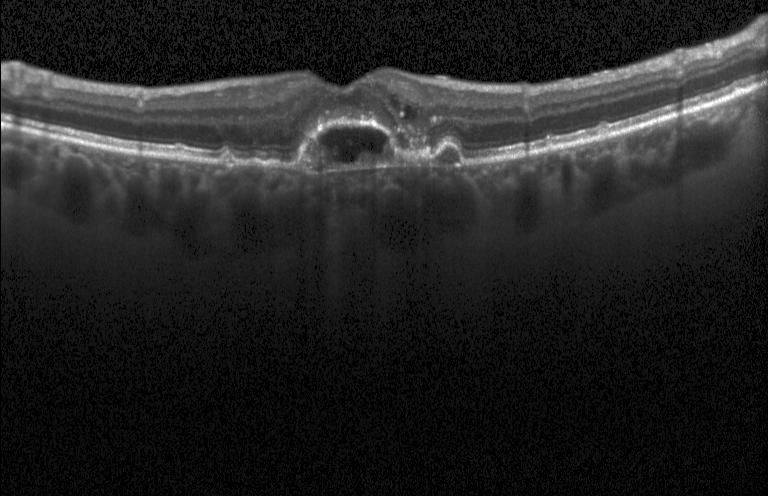 Macular scan. Instrument: Heidelberg Spectralis. Retinal OCT B-scan. Spectral-domain optical coherence tomography
Impression: a choroidal neovascular membrane.